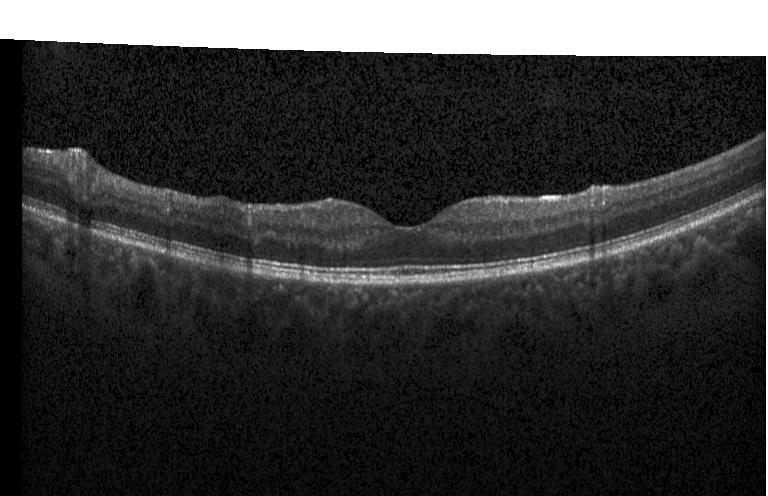
Optical coherence tomography B-scan · instrument: Heidelberg Spectralis.
Impression: neither choroidal neovascularization, diabetic macular edema, nor drusen.